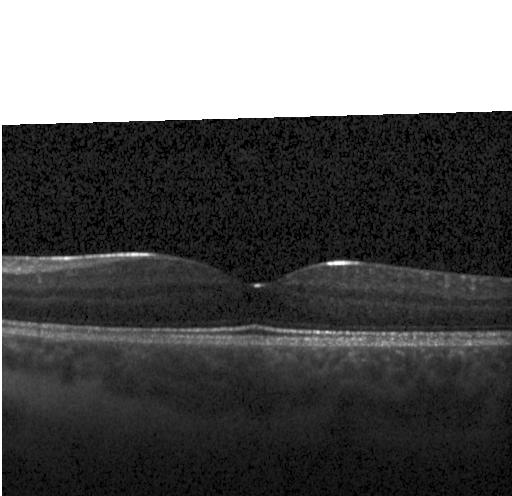
Horizontal scan through the fovea; optical coherence tomography scan; SD-OCT
This B-scan demonstrates neither choroidal neovascularization, diabetic macular edema, nor drusen.